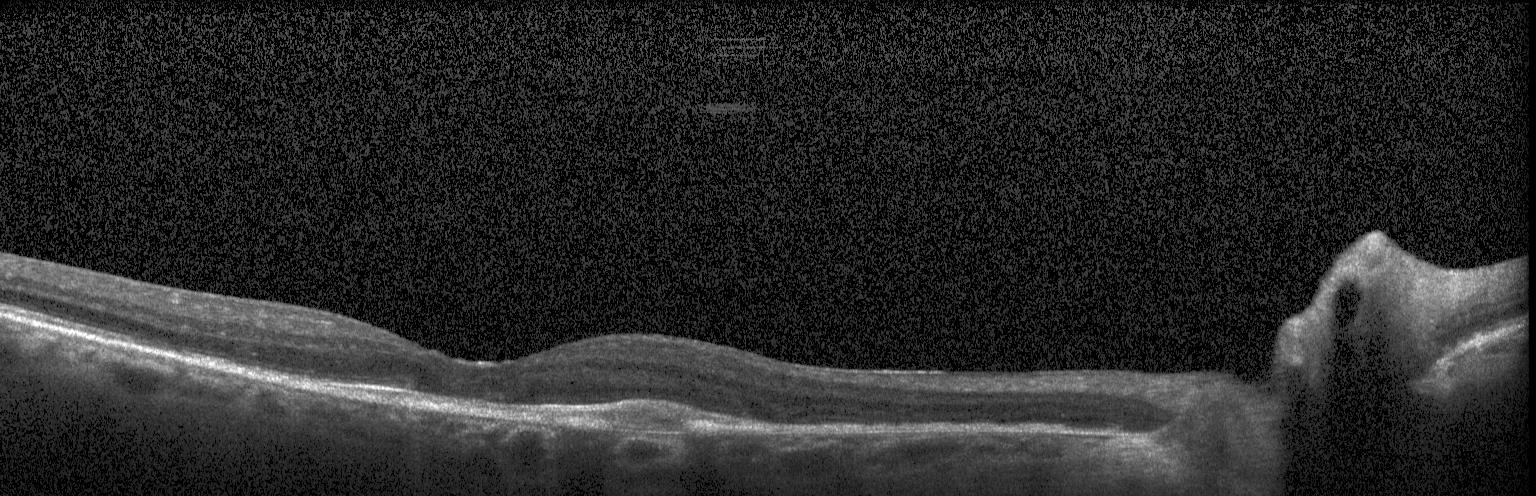

OCT B-scan
Dx: a choroidal neovascular membrane.